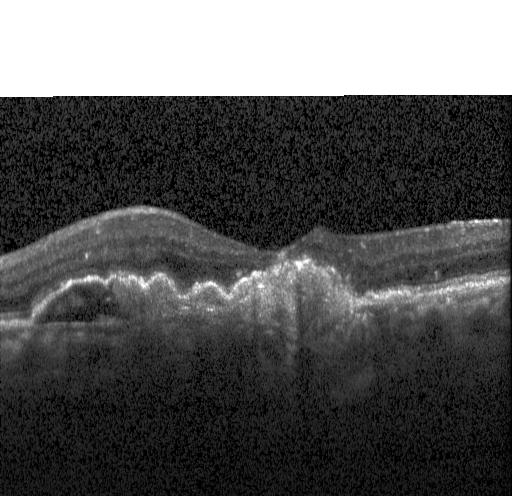
Spectral-domain OCT B-scan: a choroidal neovascular membrane.